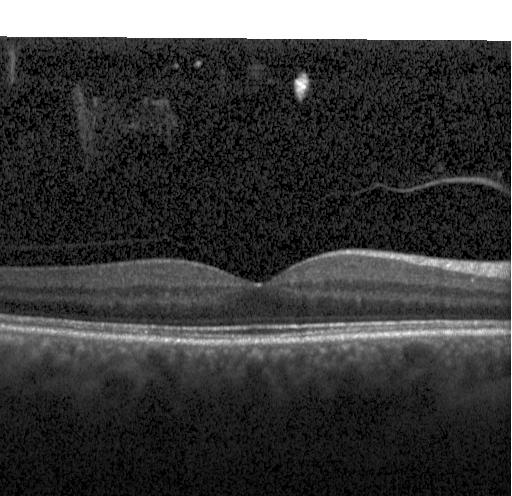 Spectral-domain OCT · OCT B-scan · Heidelberg Spectralis OCT system · fovea-centered.
Impression: no choroidal neovascularization, no diabetic macular edema, and no drusen.